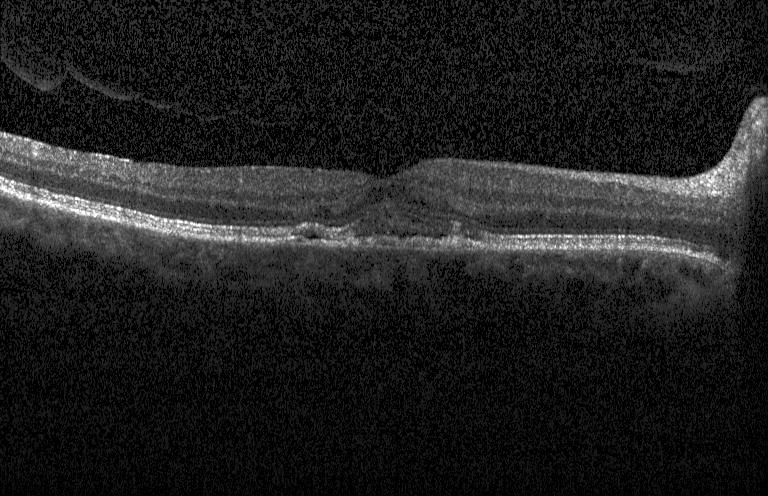
Spectral-domain OCT B-scan: a choroidal neovascular membrane.